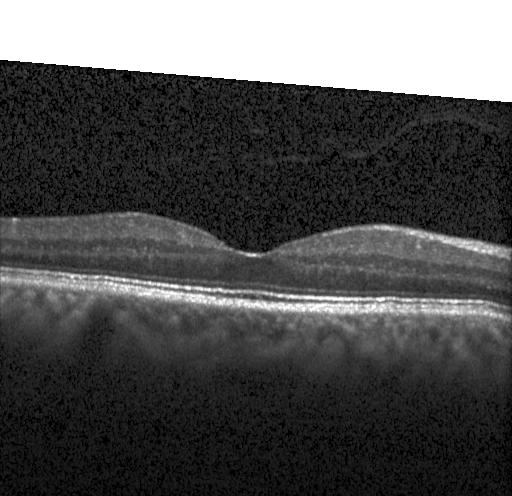

Through the macula; Heidelberg Spectralis; spectral-domain OCT; retinal OCT B-scan
The scan shows no choroidal neovascularization, diabetic macular edema, or drusen.